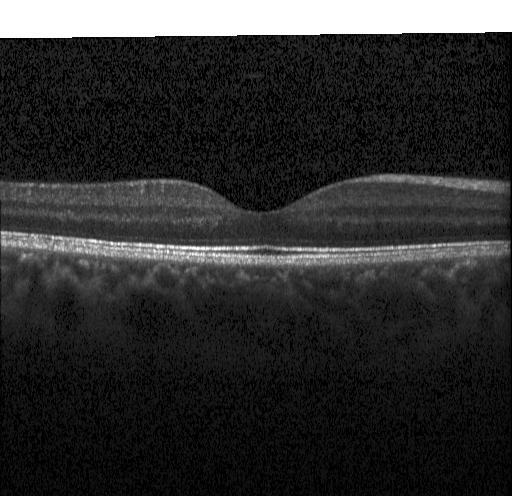

Optical coherence tomography scan. Spectral-domain optical coherence tomography. Acquired on a Heidelberg Spectralis. Horizontal scan through the fovea. Finding: no choroidal neovascularization, diabetic macular edema, or drusen.